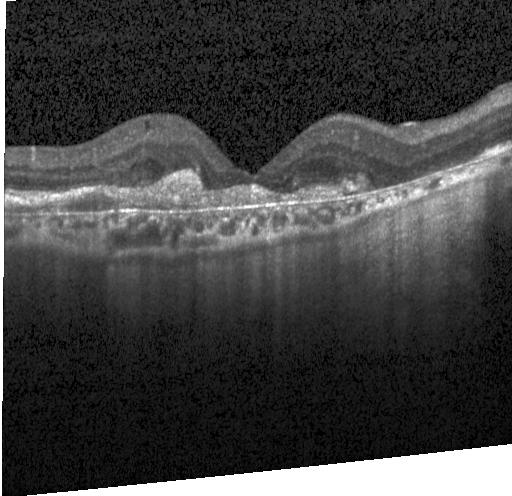
Heidelberg Spectralis, optical coherence tomography B-scan, horizontal scan through the fovea — Macular OCT: choroidal neovascularization.